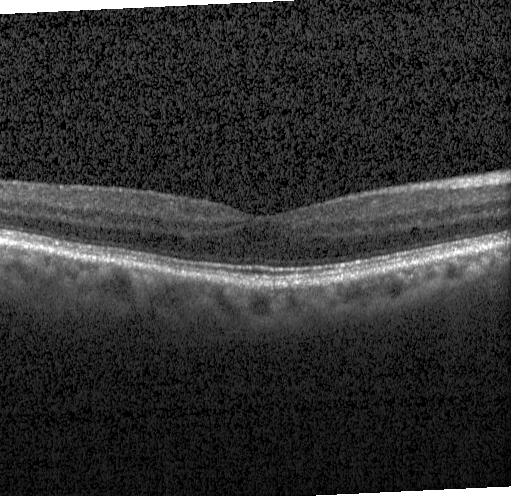

Spectral-domain OCT. Optical coherence tomography B-scan. Through the macula.
Impression: neither CNV, DME, nor drusen.